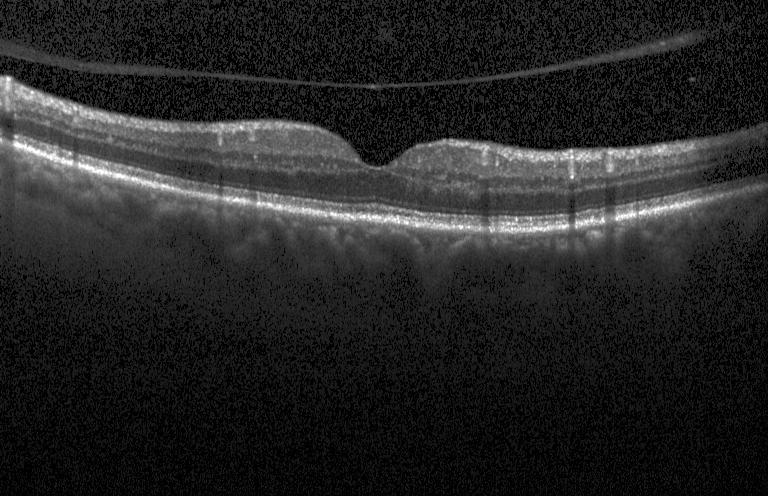 Horizontal scan through the fovea · OCT line scan · Heidelberg Spectralis OCT system. Neither CNV, DME, nor drusen.